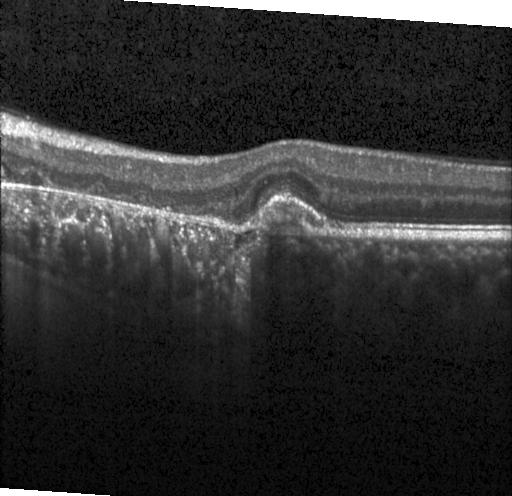

Through the macula · spectral-domain OCT · Heidelberg Spectralis · optical coherence tomography scan — Dx: a choroidal neovascular membrane.